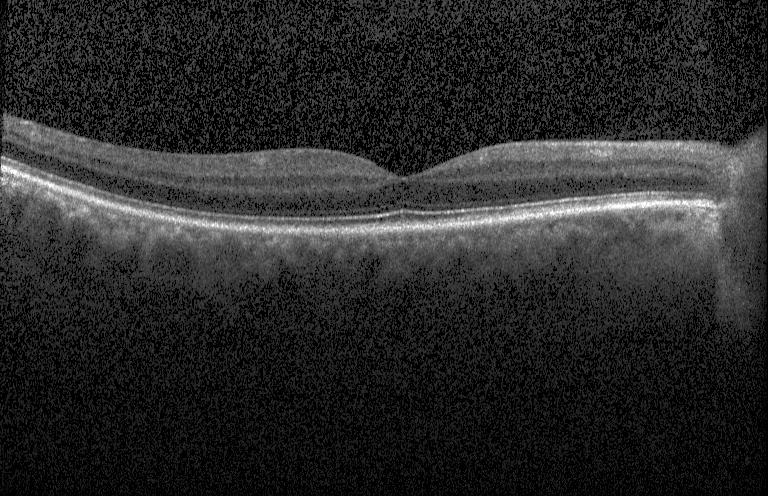

OCT line scan — OCT finding: no choroidal neovascularization, diabetic macular edema, or drusen.